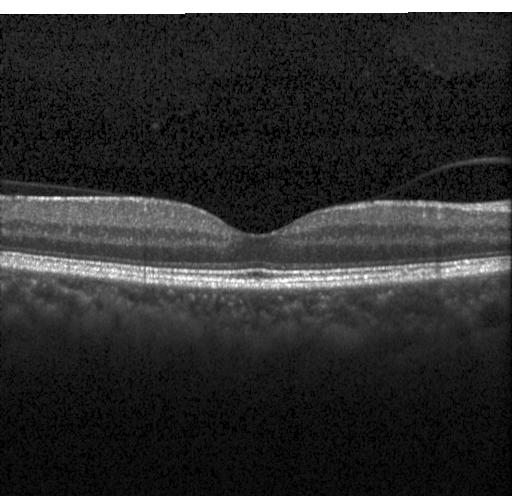
Heidelberg Spectralis OCT system; centered on the fovea; OCT line scan; spectral-domain OCT — Finding: no evidence of CNV, DME, or drusen.